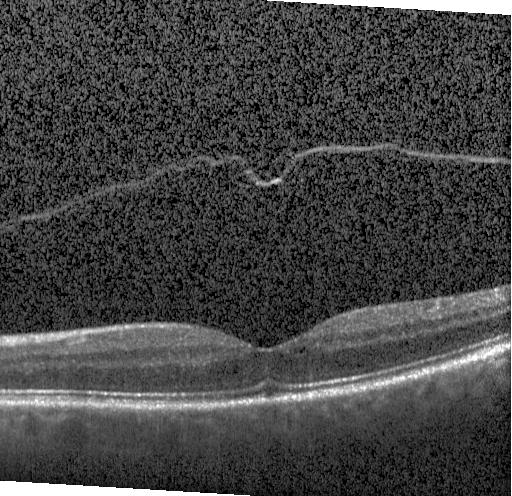
Dx: neither CNV, DME, nor drusen.